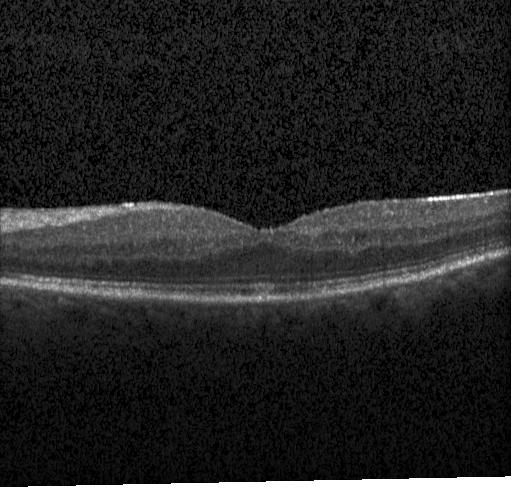 Retinal OCT B-scan. Spectral-domain optical coherence tomography.
Diagnosis: no evidence of choroidal neovascularization, diabetic macular edema, or drusen.